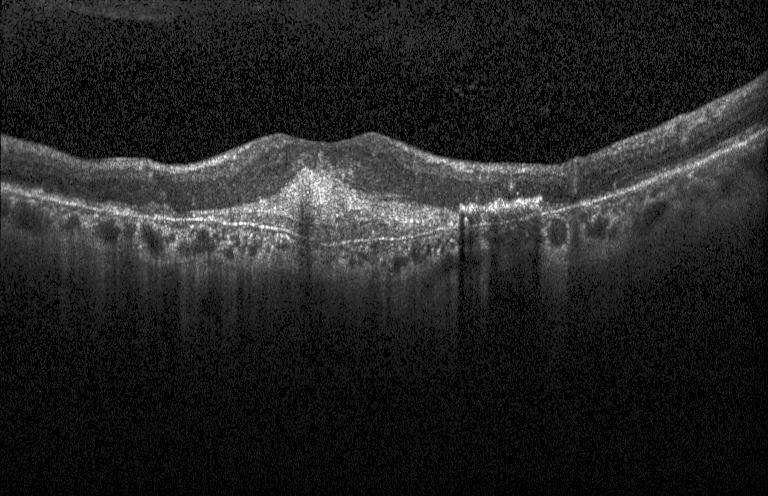 Spectral-domain OCT · acquired on a Heidelberg Spectralis · optical coherence tomography B-scan · through the macula. Choroidal neovascularization (CNV).